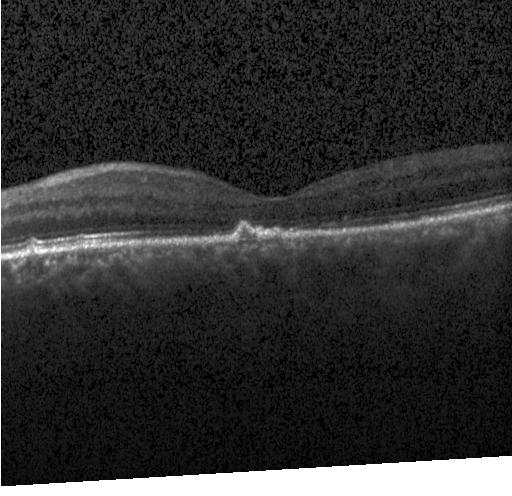 OCT finding: drusen.